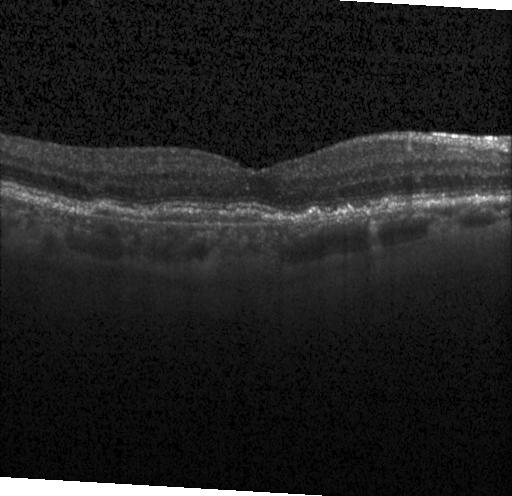 Acquired on a Heidelberg Spectralis. Spectral-domain OCT. Retinal OCT B-scan. Fovea-centered — Impression: a choroidal neovascular membrane.